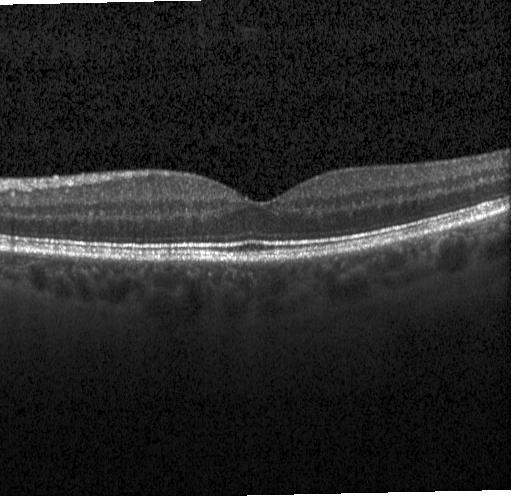 Instrument: Heidelberg Spectralis; macular scan; OCT line scan — Assessment: neither CNV, DME, nor drusen.